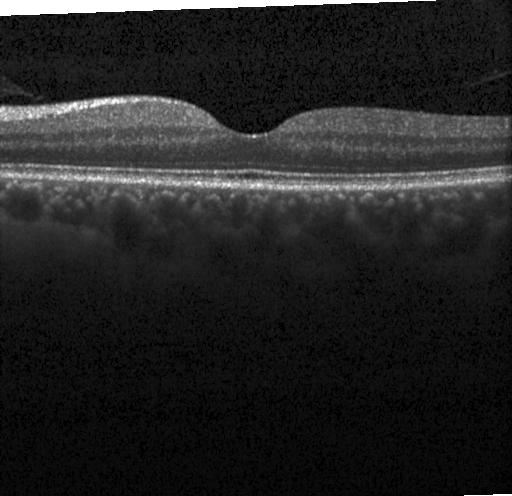

OCT finding: neither choroidal neovascularization, diabetic macular edema, nor drusen.